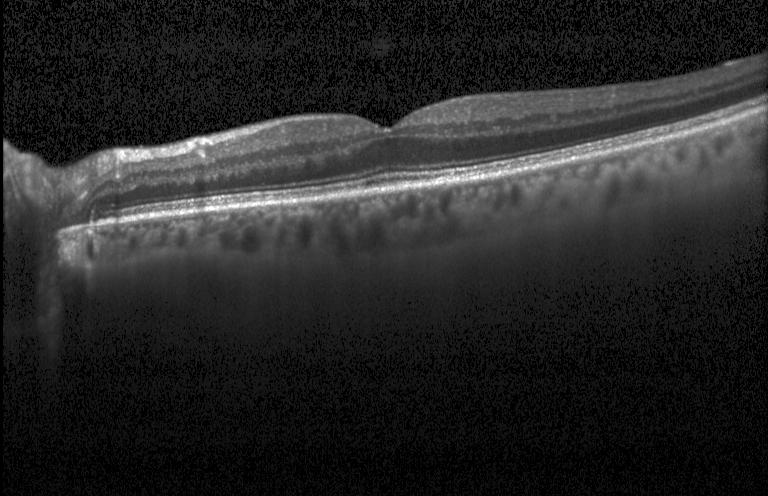 Diagnosis: no choroidal neovascularization, no diabetic macular edema, and no drusen.